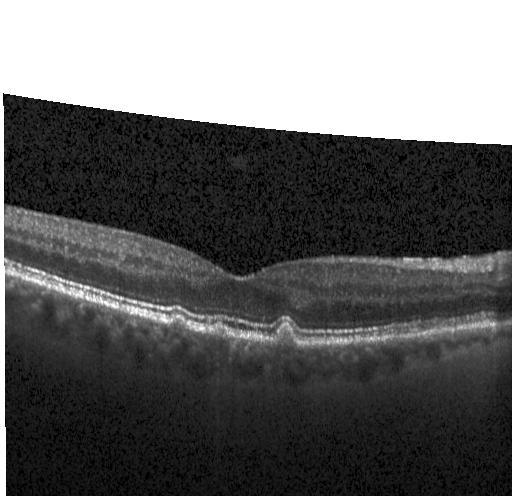
OCT B-scan showing drusen.